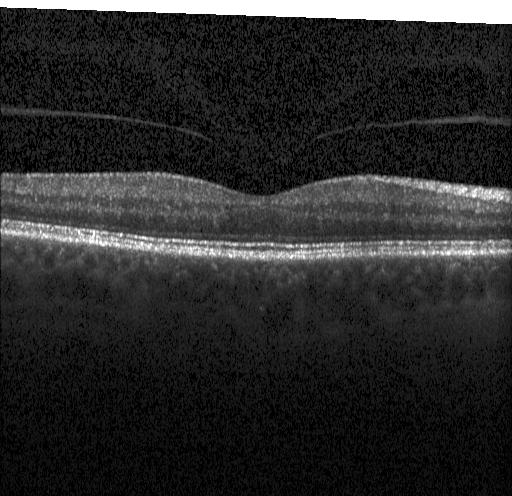
Assessment: no choroidal neovascularization, diabetic macular edema, or drusen.